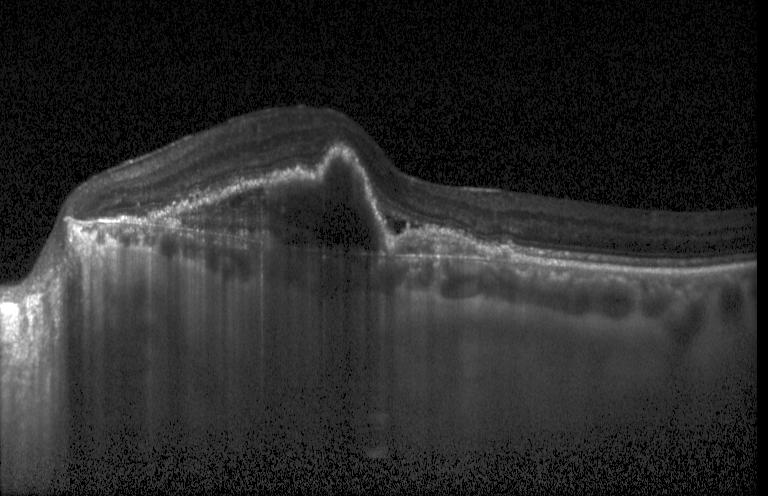
Impression: CNV.